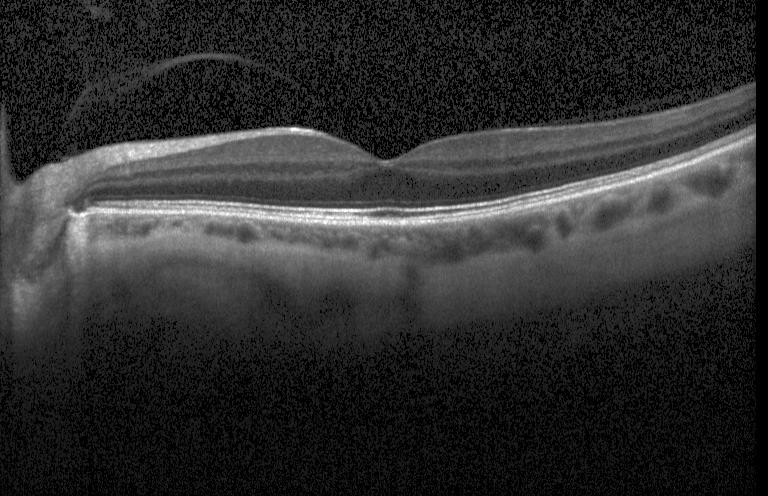
OCT B-scan showing neither CNV, DME, nor drusen.